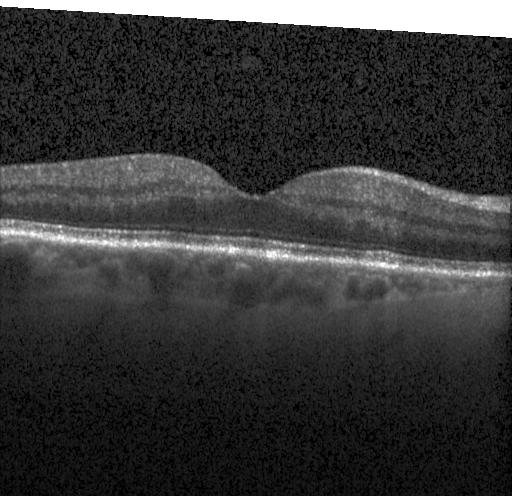

Dx: neither CNV, DME, nor drusen.